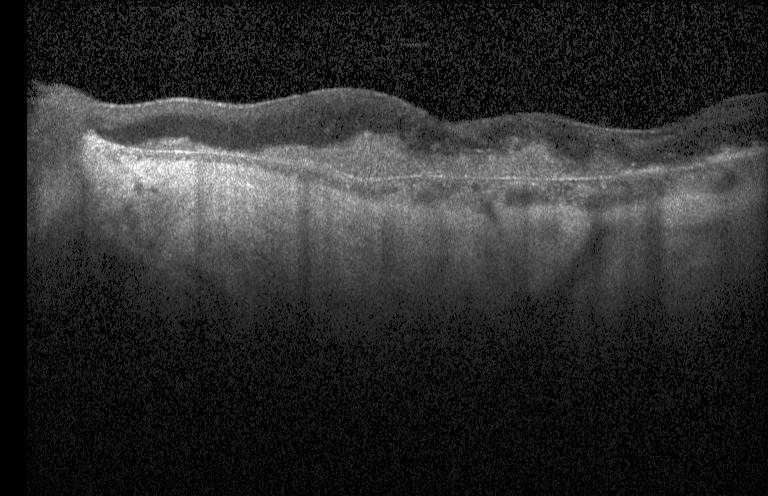

Spectral-domain OCT · retinal OCT B-scan · horizontal scan through the fovea · instrument: Heidelberg Spectralis.
Assessment: a choroidal neovascular membrane.